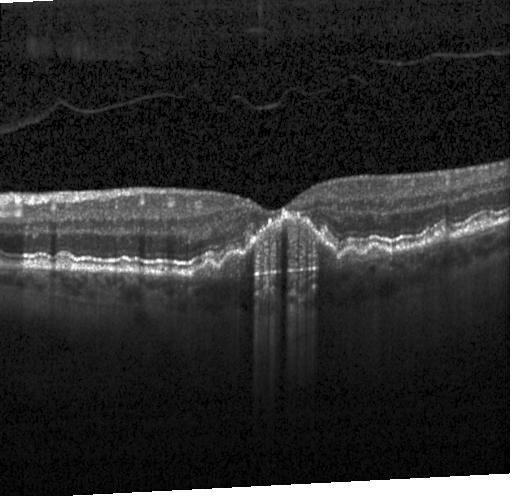

Macular scan. SD-OCT. Heidelberg Spectralis. OCT line scan — Finding: a choroidal neovascular membrane.